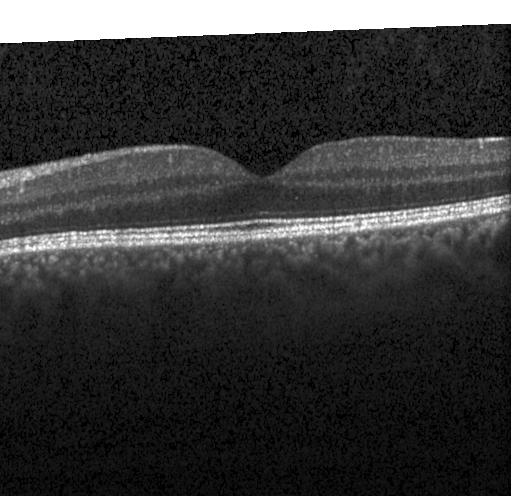

No evidence of choroidal neovascularization, diabetic macular edema, or drusen.